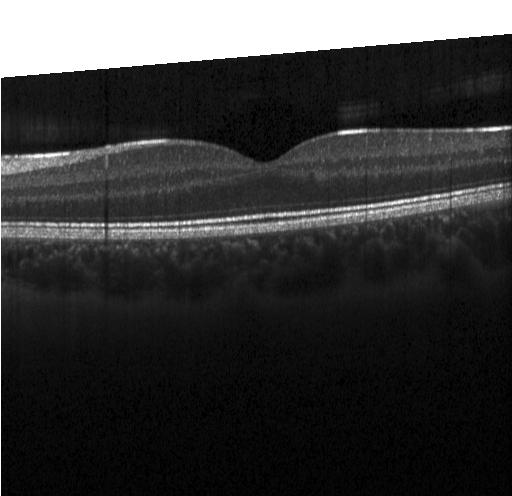 Spectral-domain OCT B-scan: no evidence of choroidal neovascularization, diabetic macular edema, or drusen.